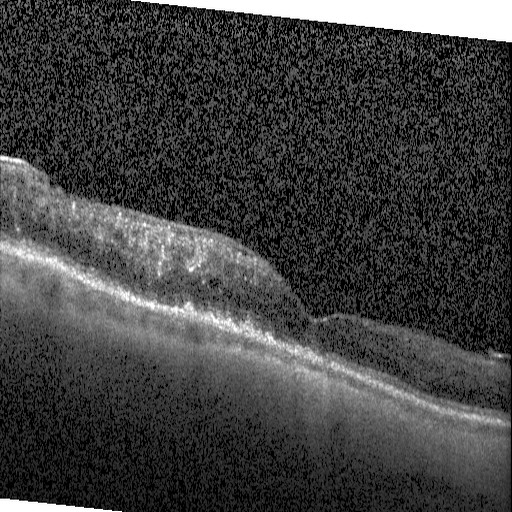
Diagnosis: diabetic macular edema.